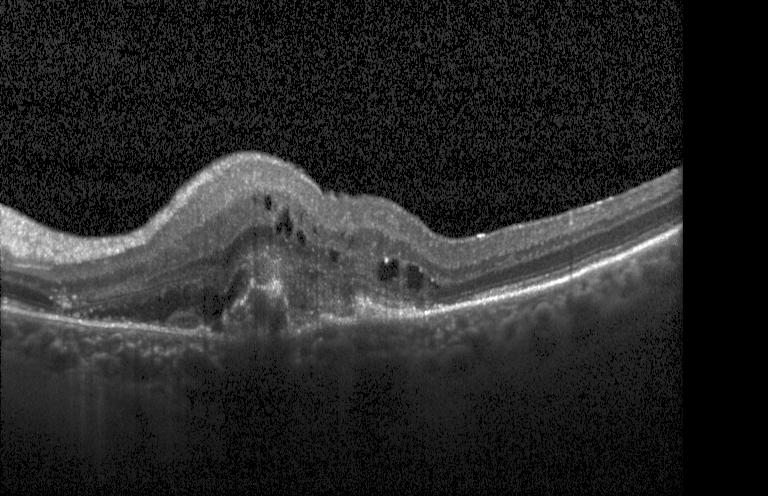
Retinal OCT cross-section
Finding: CNV.